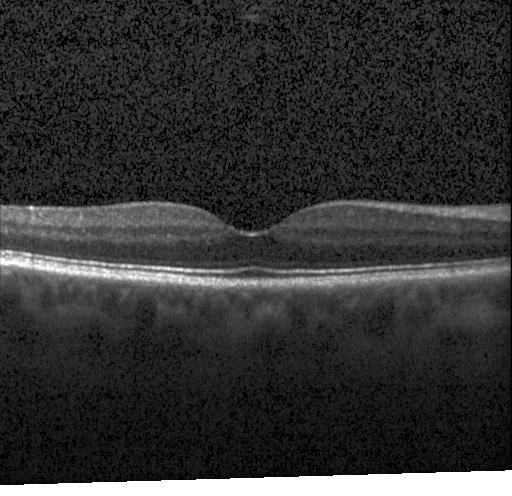 OCT B-scan. Impression: no evidence of choroidal neovascularization, diabetic macular edema, or drusen.